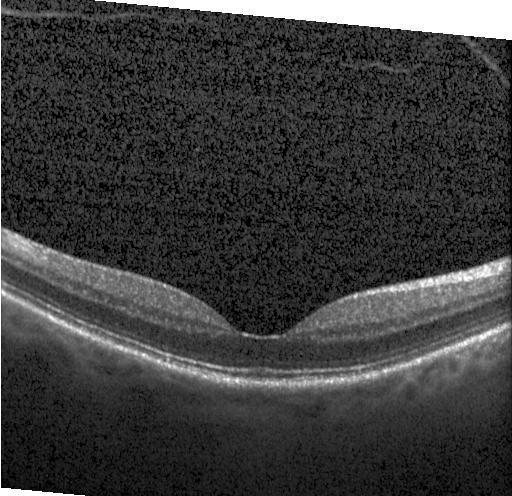 OCT scan showing no CNV, no DME, and no drusen.